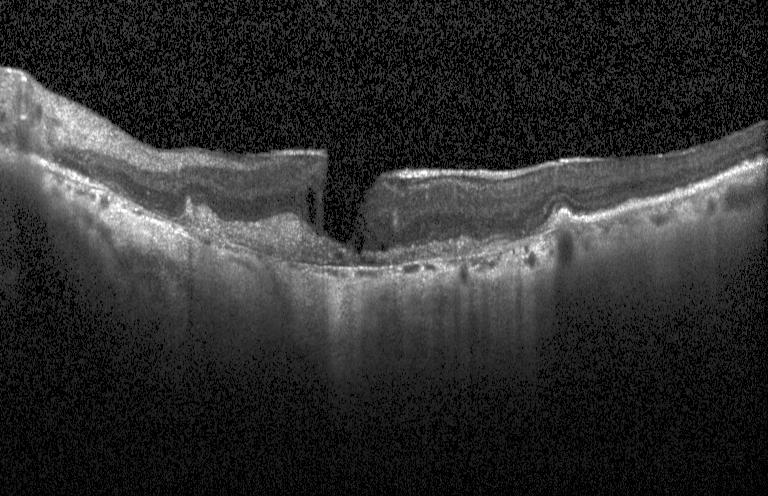 Macular scan · Heidelberg Spectralis OCT system · optical coherence tomography B-scan · spectral-domain optical coherence tomography
Macular OCT: a choroidal neovascular membrane.